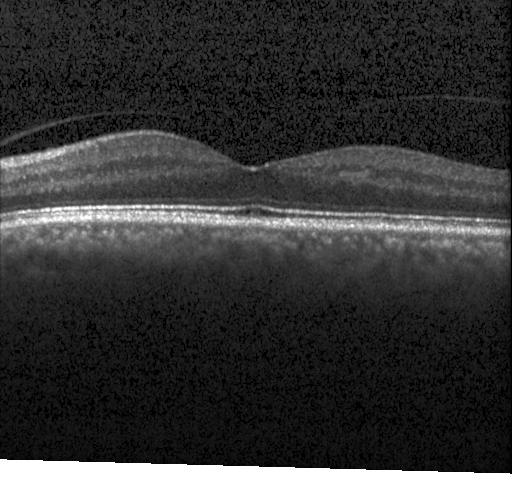
Instrument: Heidelberg Spectralis, retinal OCT B-scan.
The scan shows no evidence of choroidal neovascularization, diabetic macular edema, or drusen.